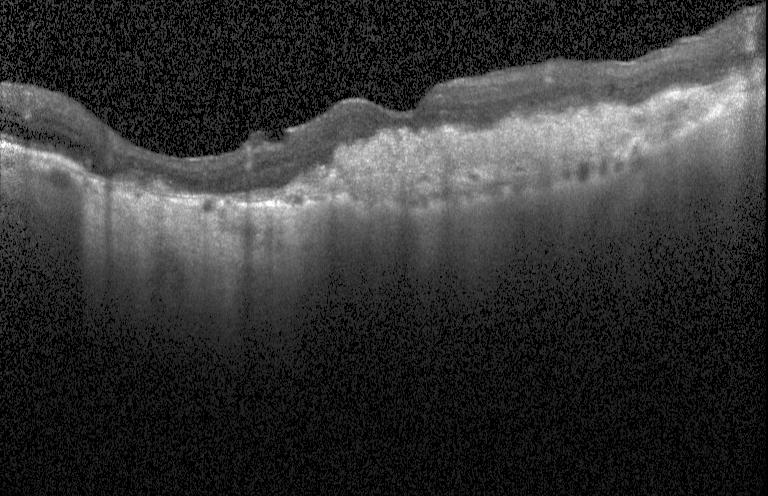

OCT finding: choroidal neovascularization (CNV).